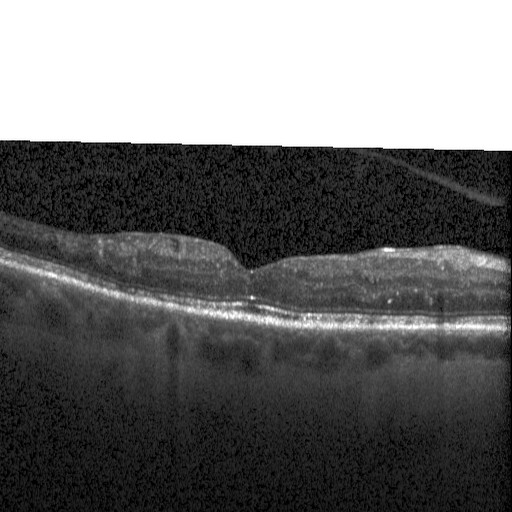 Diagnosis: DME.